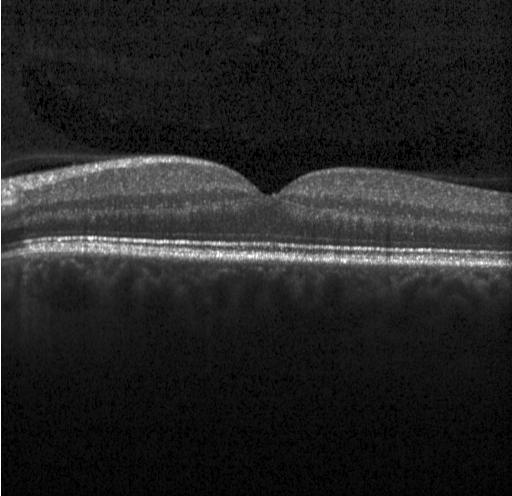
No evidence of CNV, DME, or drusen.